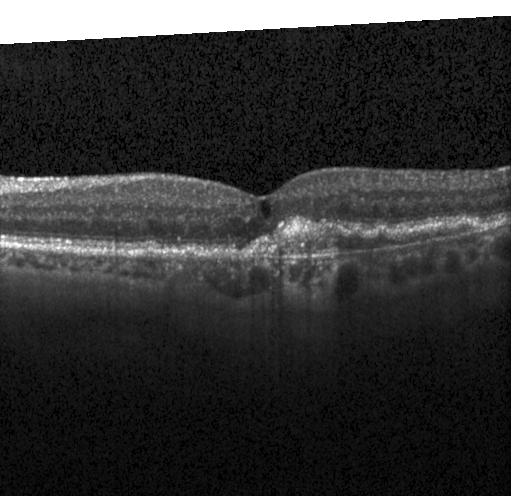

Finding: CNV.